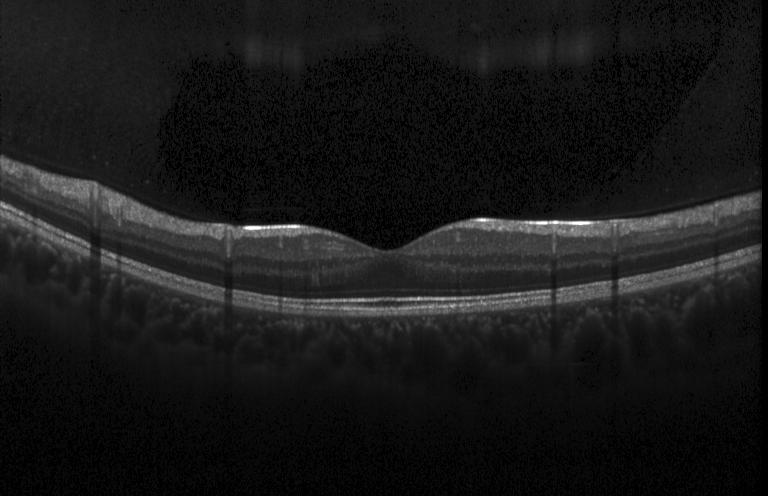
Spectral-domain OCT B-scan: no evidence of choroidal neovascularization, diabetic macular edema, or drusen.